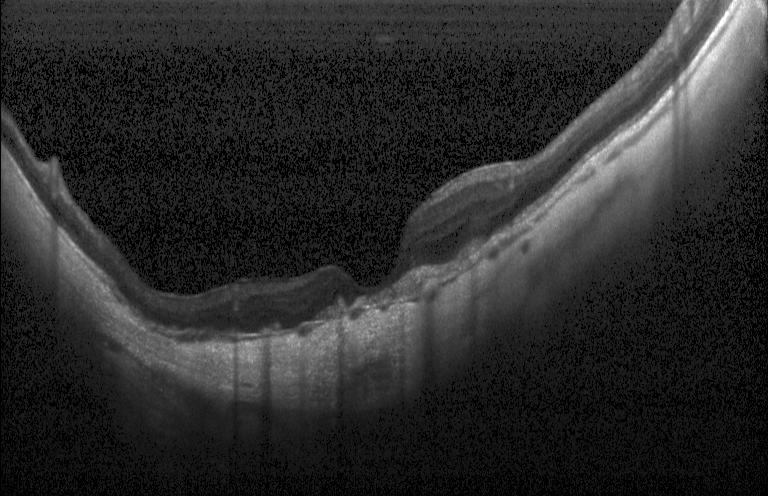
OCT finding: choroidal neovascularization (CNV).